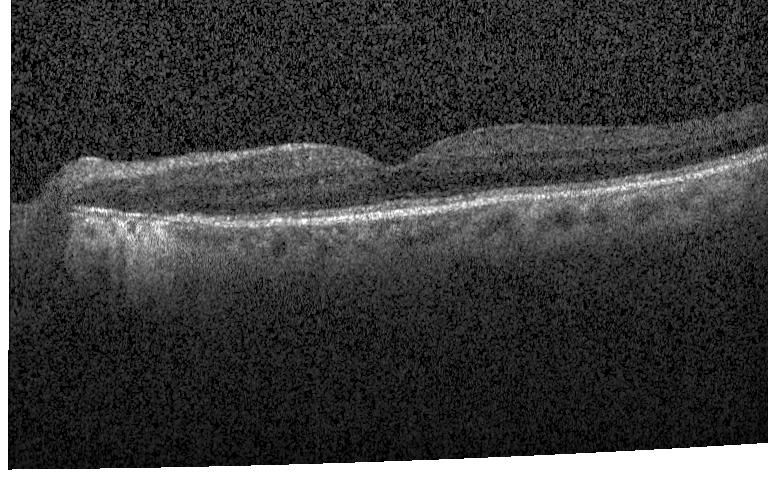

Retinal OCT cross-section · SD-OCT. Diagnosis: no evidence of choroidal neovascularization, diabetic macular edema, or drusen.